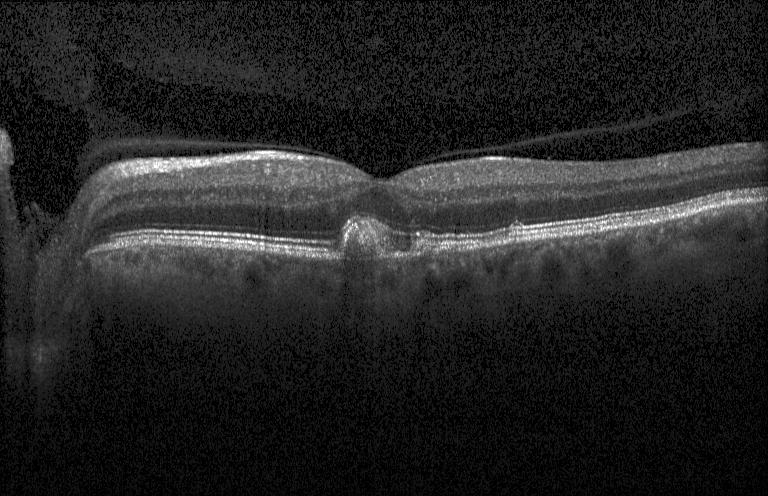
Macular OCT demonstrating sub-RPE drusenoid deposits.